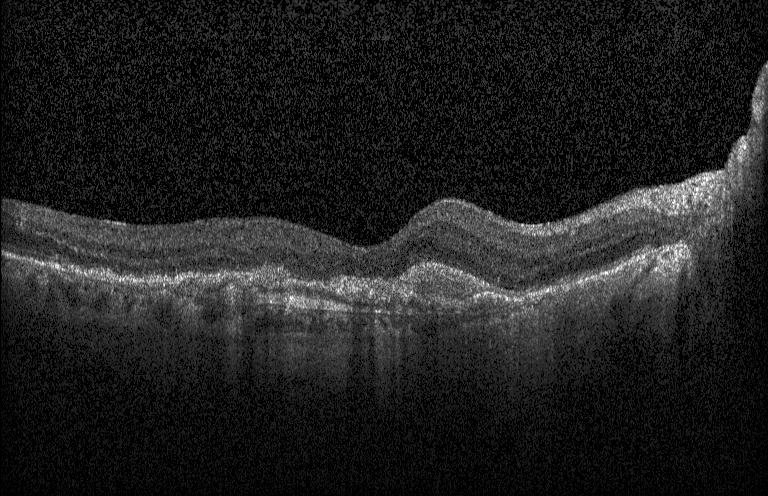

Macular OCT demonstrating a choroidal neovascular membrane.